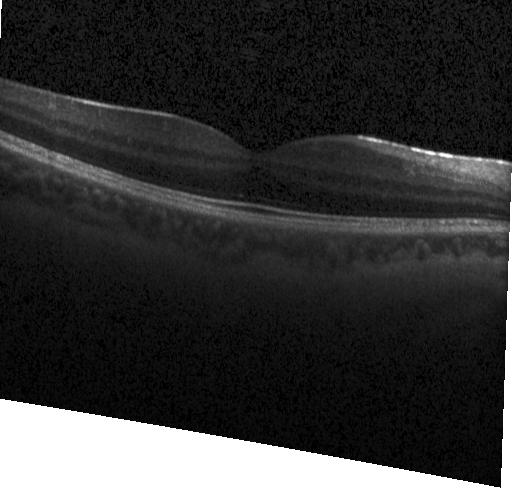
Retinal OCT B-scan.
Finding: no evidence of choroidal neovascularization, diabetic macular edema, or drusen.